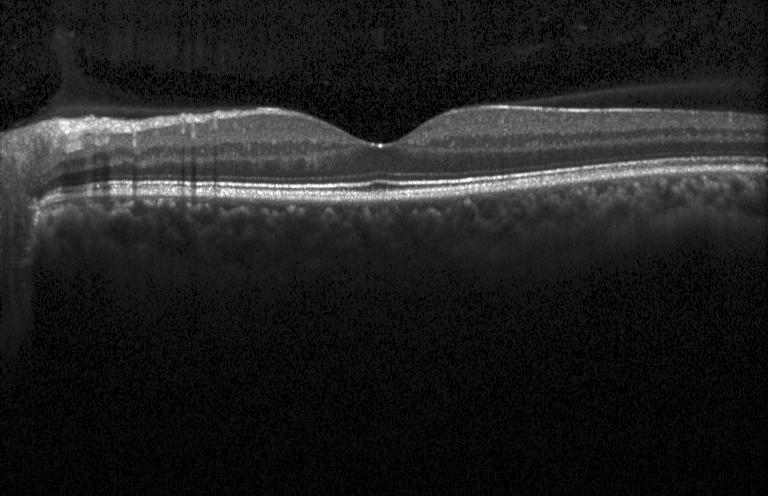
Optical coherence tomography scan · spectral-domain OCT · fovea-centered · instrument: Heidelberg Spectralis.
This B-scan demonstrates no choroidal neovascularization, no diabetic macular edema, and no drusen.